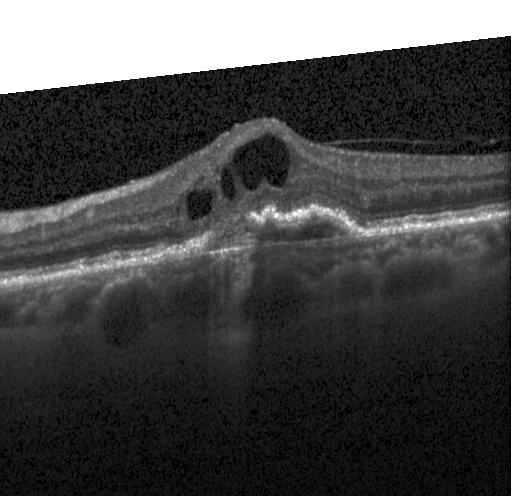 Retinal OCT cross-section
Finding: a choroidal neovascular membrane.